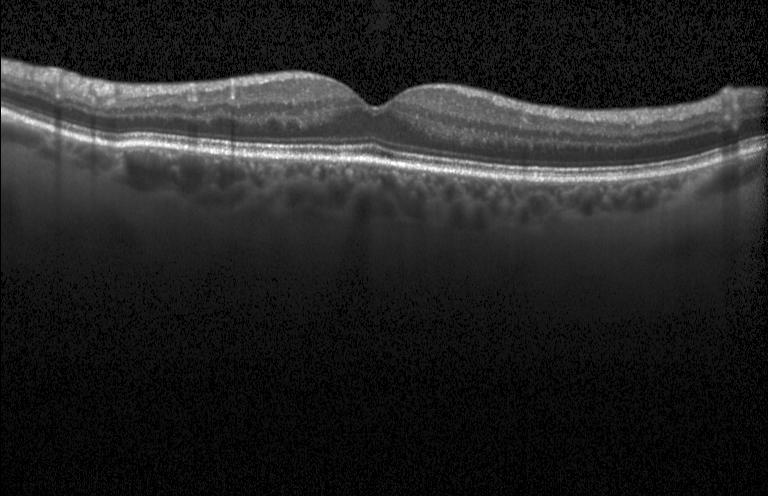

OCT line scan. Spectral-domain OCT — OCT finding: neither choroidal neovascularization, diabetic macular edema, nor drusen.